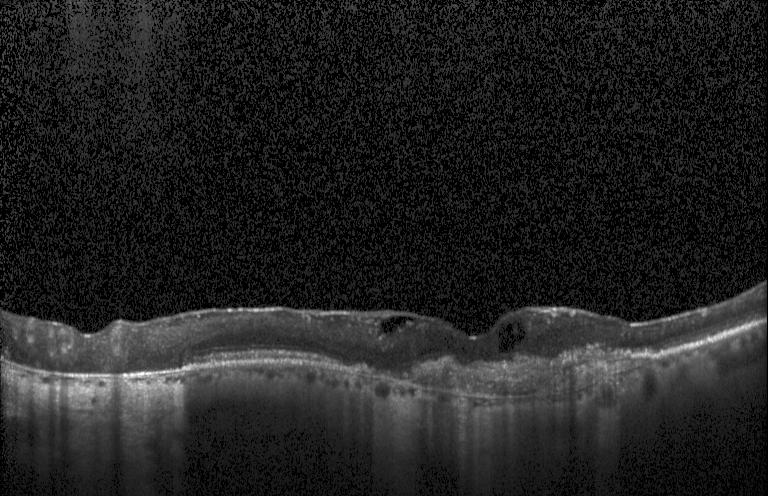

SD-OCT; optical coherence tomography scan
Diagnosis: a choroidal neovascular membrane.